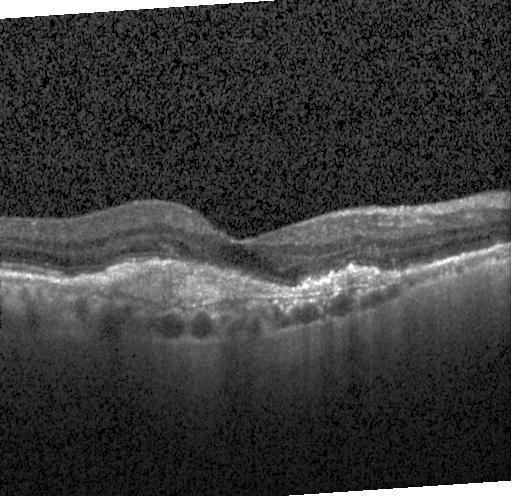 OCT line scan. OCT finding: a choroidal neovascular membrane.